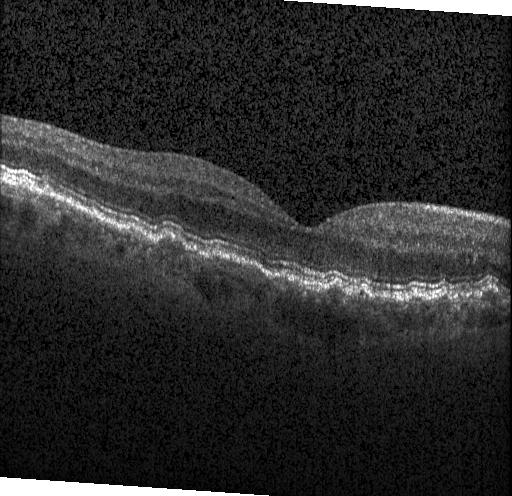
Fovea-centered; retinal OCT B-scan; spectral-domain optical coherence tomography — Finding: multiple drusen.